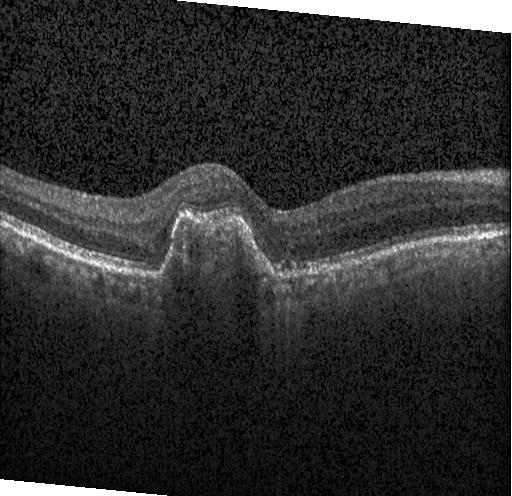 OCT B-scan. Macular scan. Instrument: Heidelberg Spectralis
Diagnosis: choroidal neovascularization (CNV).